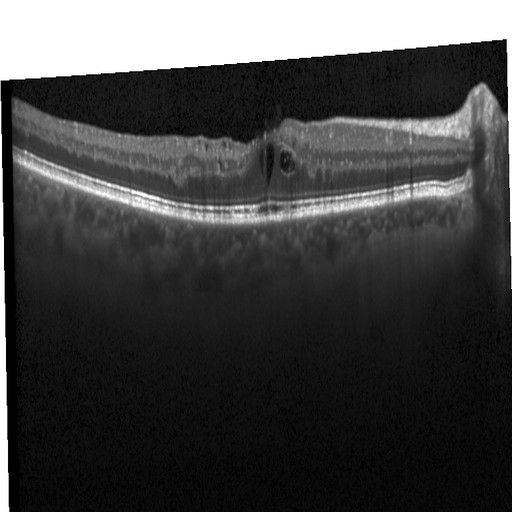 Optical coherence tomography scan, spectral-domain optical coherence tomography, instrument: Heidelberg Spectralis, horizontal scan through the fovea
Diagnosis: diabetic macular edema.